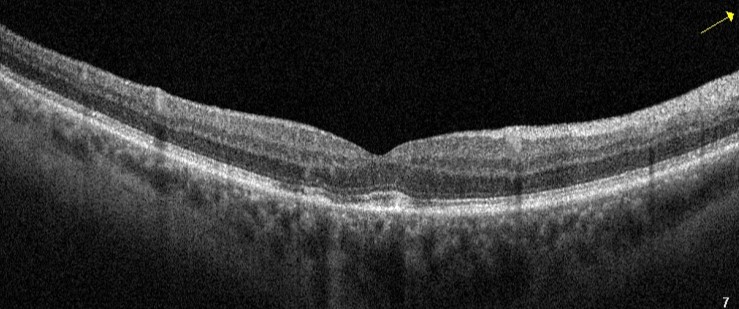 Retinal OCT B-scan.
This B-scan demonstrates age-related macular degeneration.